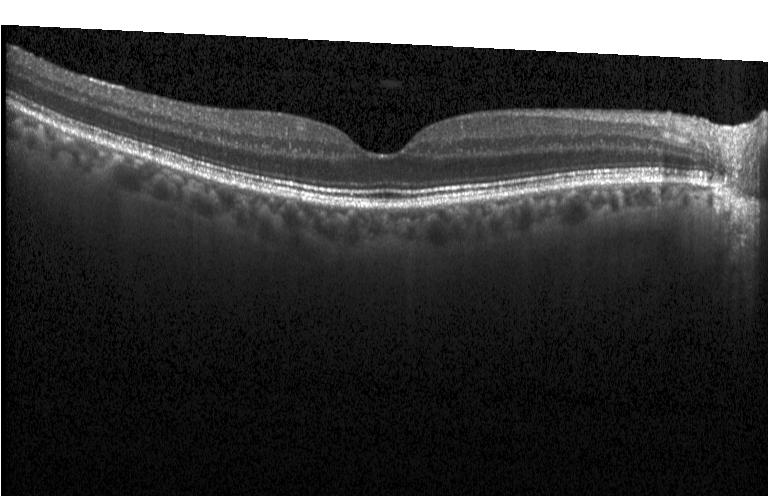 OCT line scan; fovea-centered
Finding: no choroidal neovascularization, diabetic macular edema, or drusen.